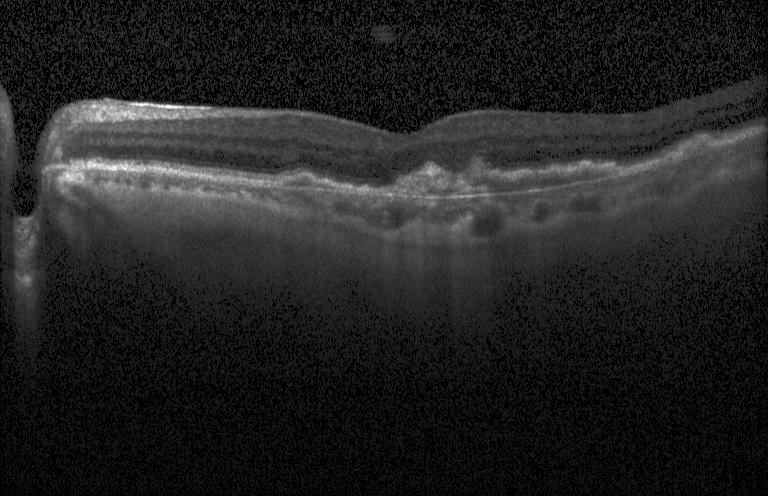 Optical coherence tomography B-scan · spectral-domain OCT · acquired on a Heidelberg Spectralis · horizontal scan through the fovea — Assessment: choroidal neovascularization (CNV).